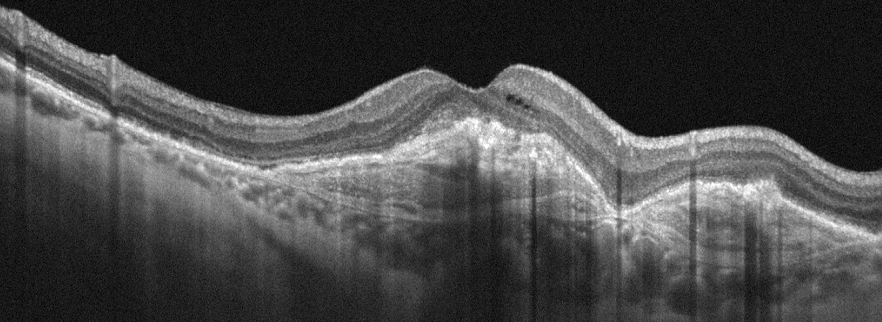

Macular scan, retinal OCT cross-section, instrument: Optovue Avanti RTVue XR
Diagnosis: AMD.